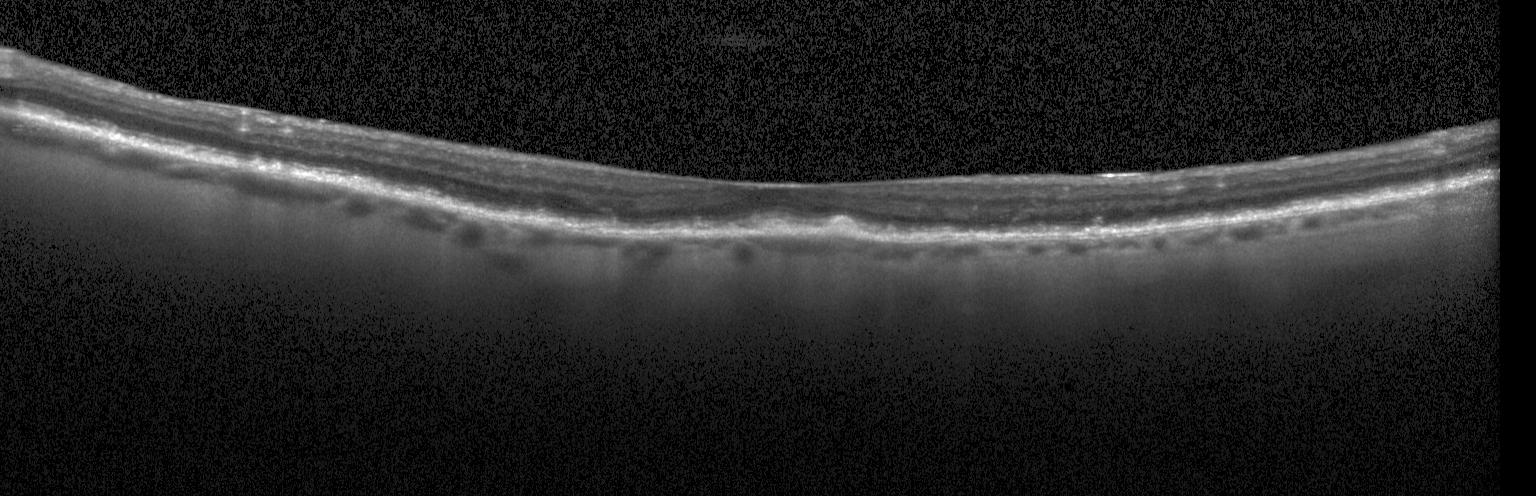

Macular OCT demonstrating CNV.